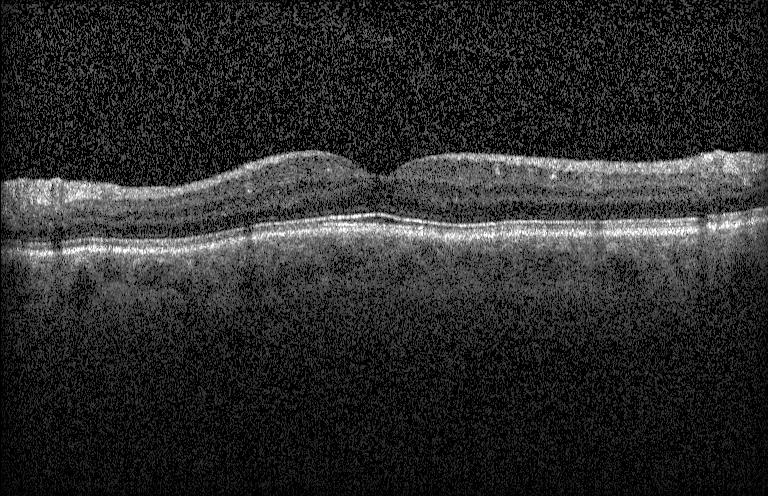
OCT finding: no CNV, no DME, and no drusen.